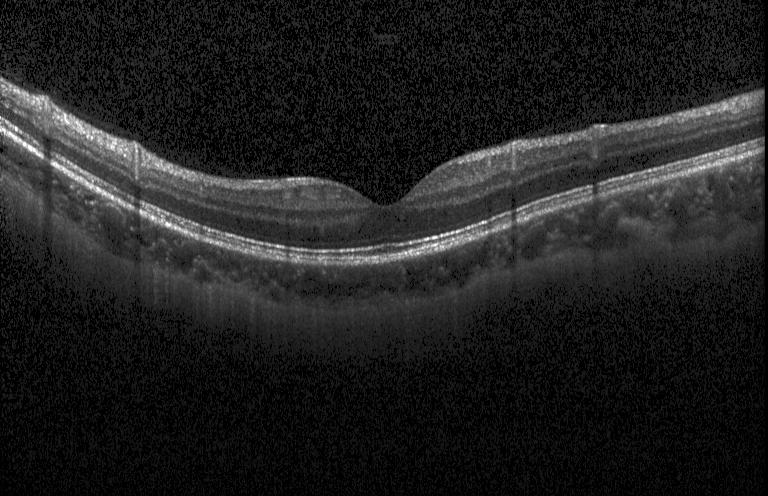 Optical coherence tomography B-scan
Impression: no choroidal neovascularization, diabetic macular edema, or drusen.